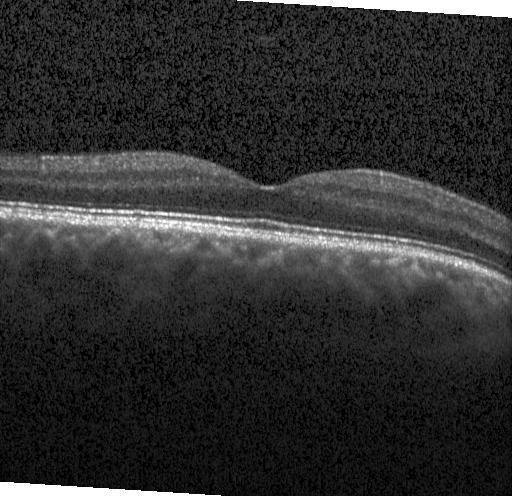

SD-OCT · acquired on a Heidelberg Spectralis · fovea-centered · OCT B-scan. Impression: no CNV, DME, or drusen.